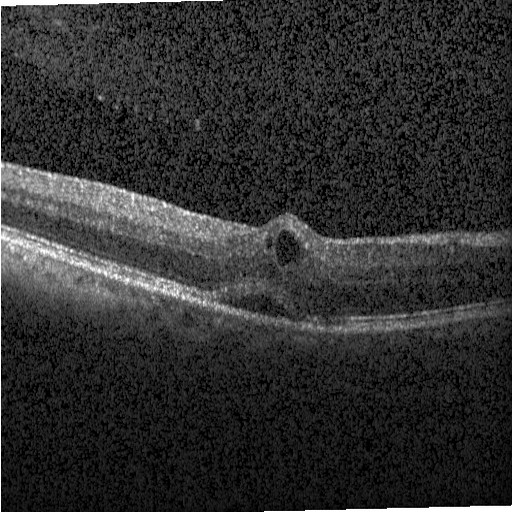 Assessment: diabetic macular edema (DME).